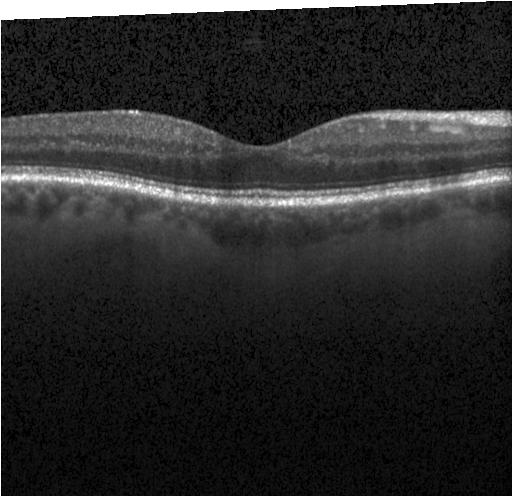 Spectral-domain optical coherence tomography; retinal OCT cross-section; through the macula; Heidelberg Spectralis OCT system — This B-scan demonstrates no choroidal neovascularization, no diabetic macular edema, and no drusen.